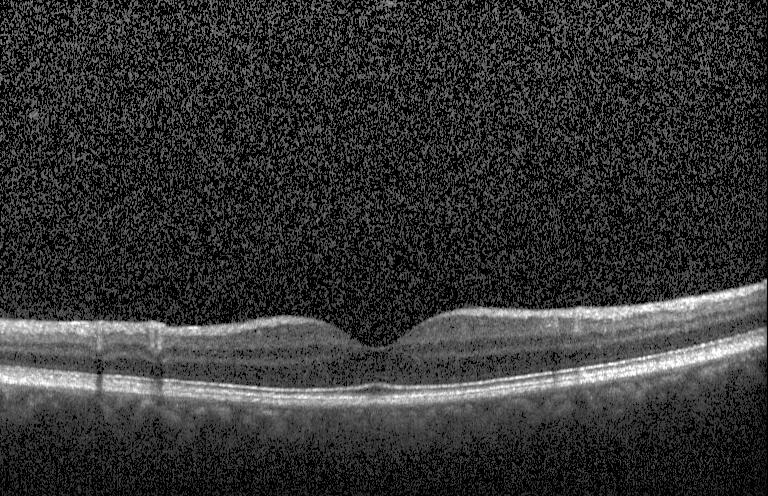

Macular OCT: no evidence of choroidal neovascularization, diabetic macular edema, or drusen.